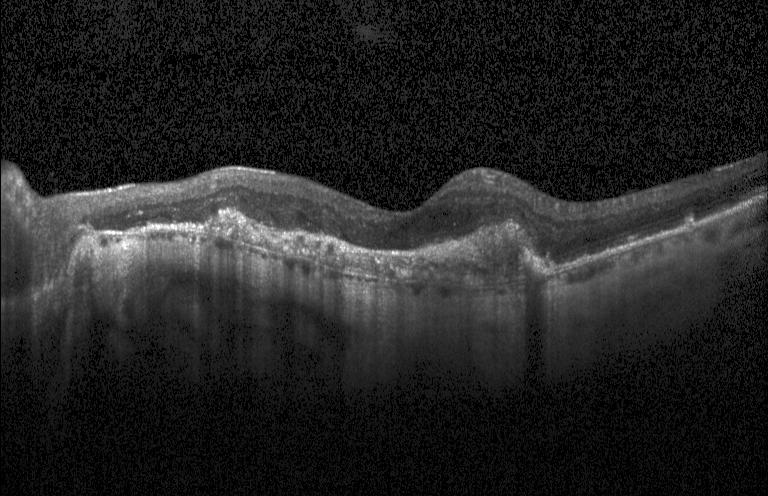
Choroidal neovascularization.